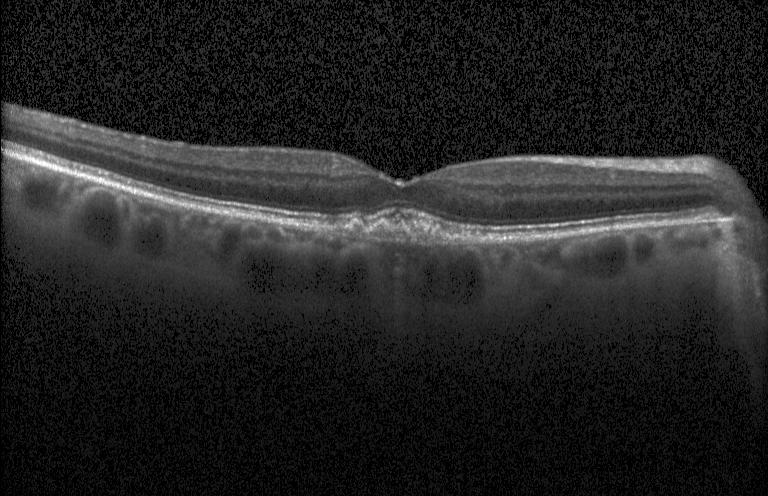
The scan shows multiple drusen.